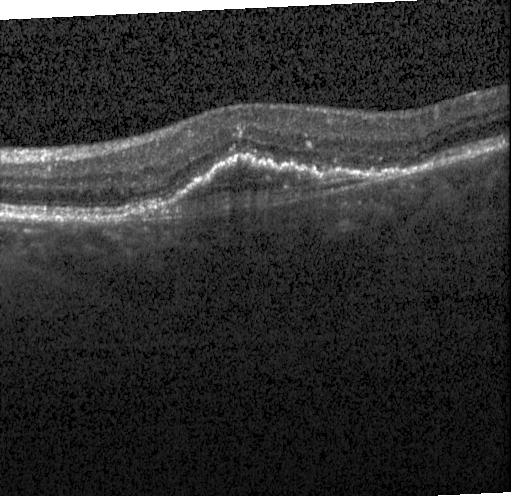 Retinal OCT cross-section — Assessment: a choroidal neovascular membrane.